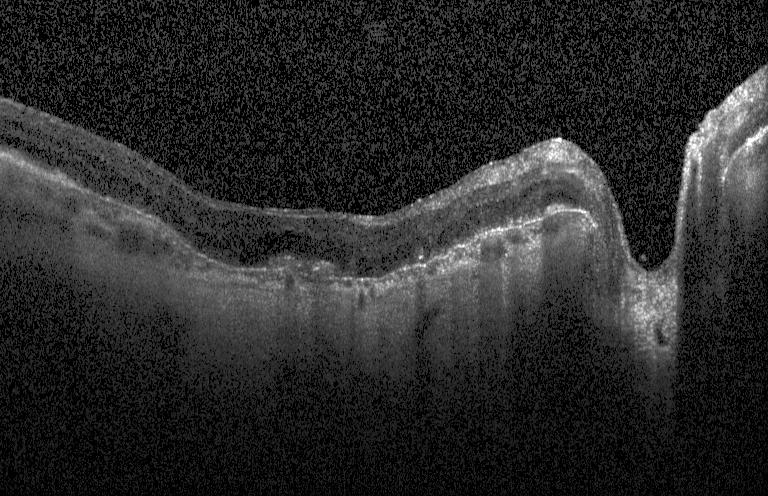 Horizontal scan through the fovea, Heidelberg Spectralis, optical coherence tomography B-scan
This B-scan demonstrates a choroidal neovascular membrane.